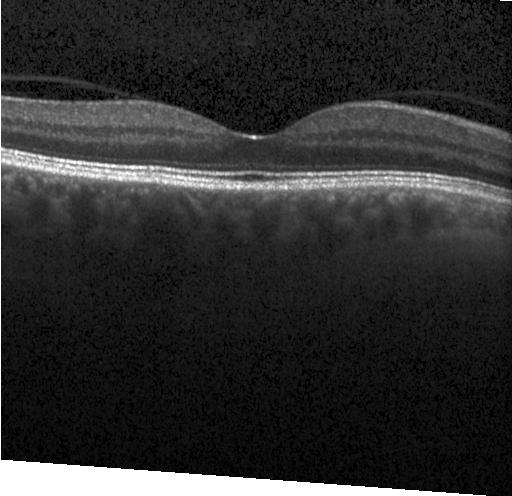

The scan shows no evidence of CNV, DME, or drusen.